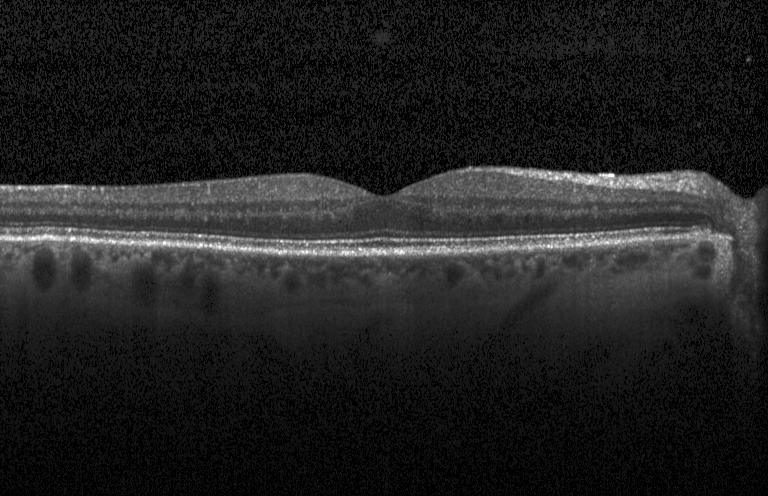
Spectral-domain optical coherence tomography; through the macula; optical coherence tomography B-scan; Heidelberg Spectralis OCT system. Diagnosis: neither choroidal neovascularization, diabetic macular edema, nor drusen.